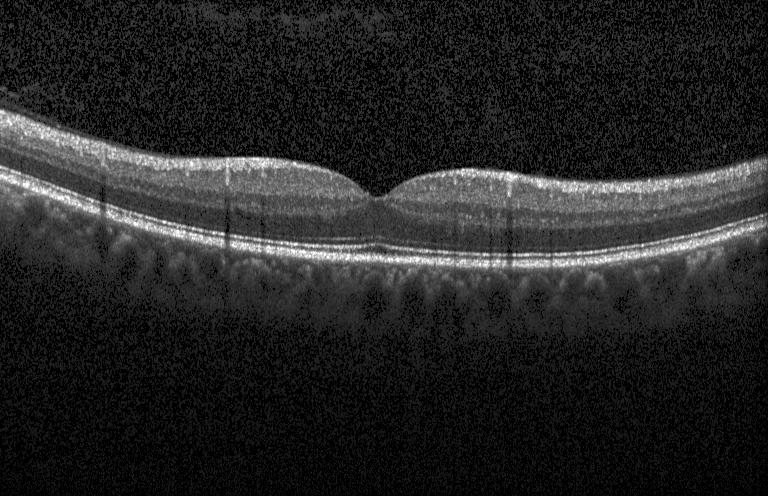
Retinal OCT cross-section showing neither CNV, DME, nor drusen.